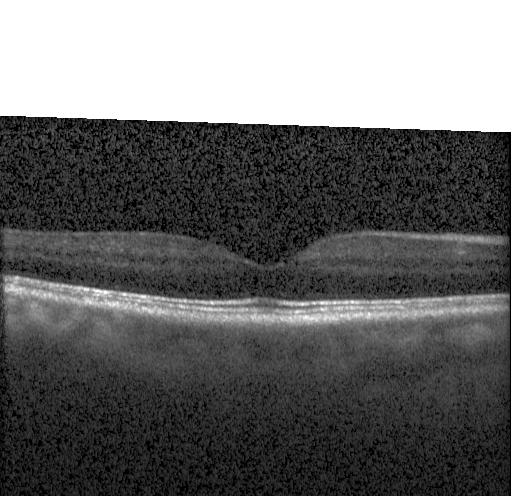
Optical coherence tomography scan.
Impression: no CNV, DME, or drusen.